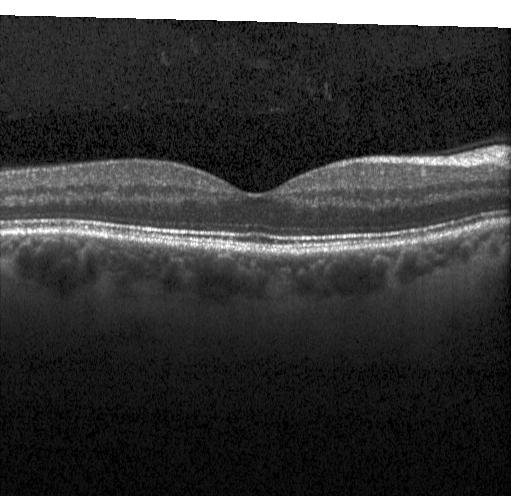

Retinal OCT cross-section. Finding: no evidence of choroidal neovascularization, diabetic macular edema, or drusen.